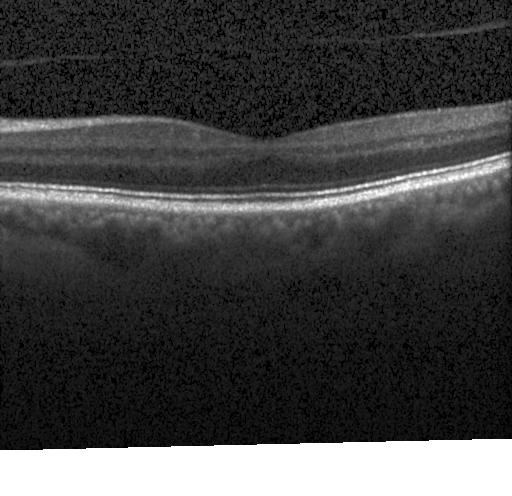
OCT B-scan, centered on the fovea.
OCT finding: no choroidal neovascularization, diabetic macular edema, or drusen.